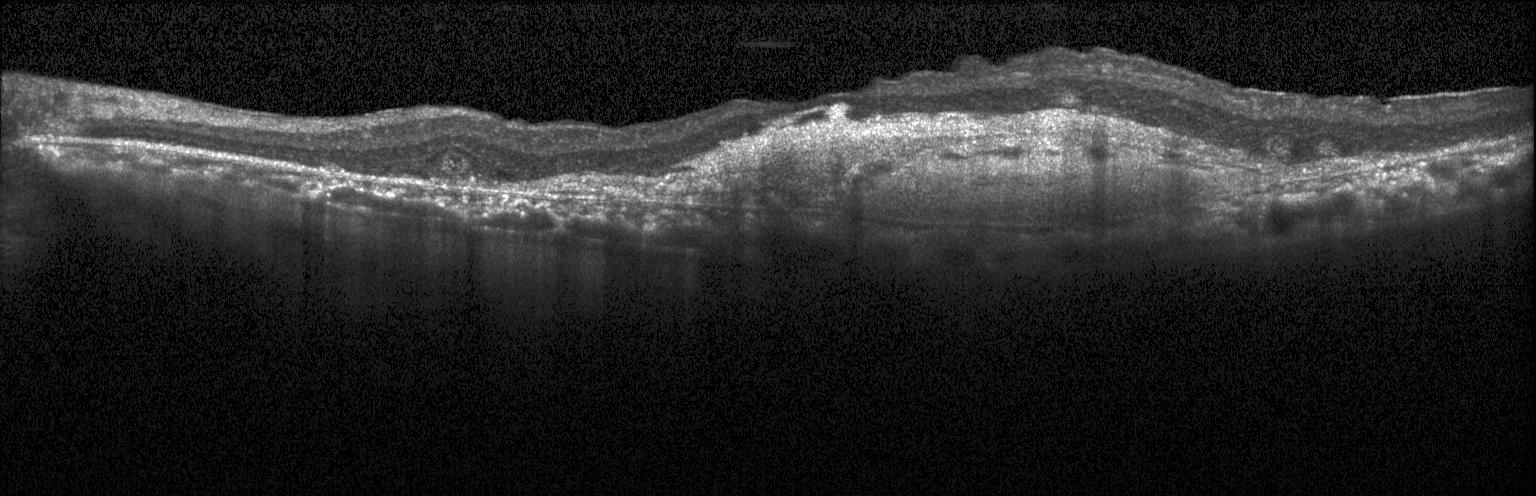

Spectral-domain OCT B-scan: a choroidal neovascular membrane.